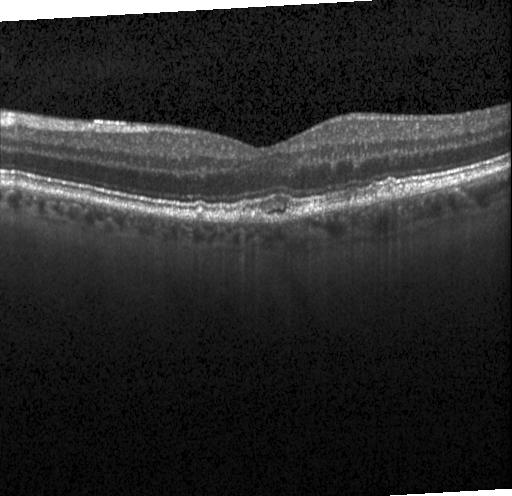

Impression: choroidal neovascularization.